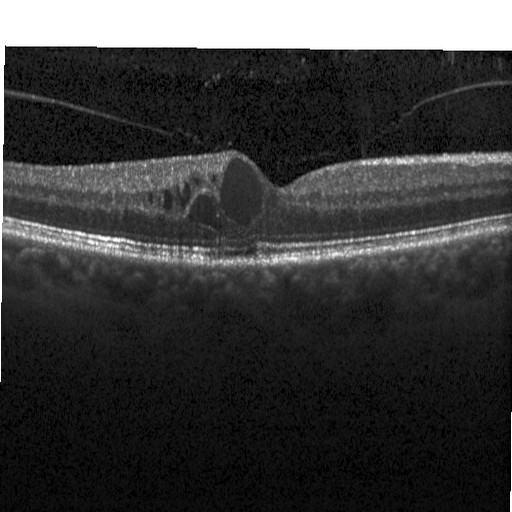 The scan shows diabetic macular edema.